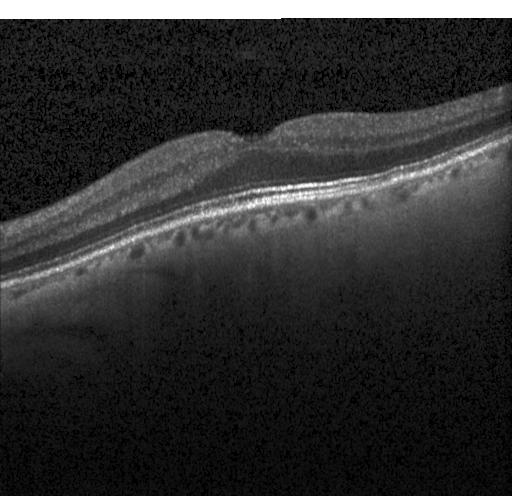

Impression: no CNV, no DME, and no drusen.